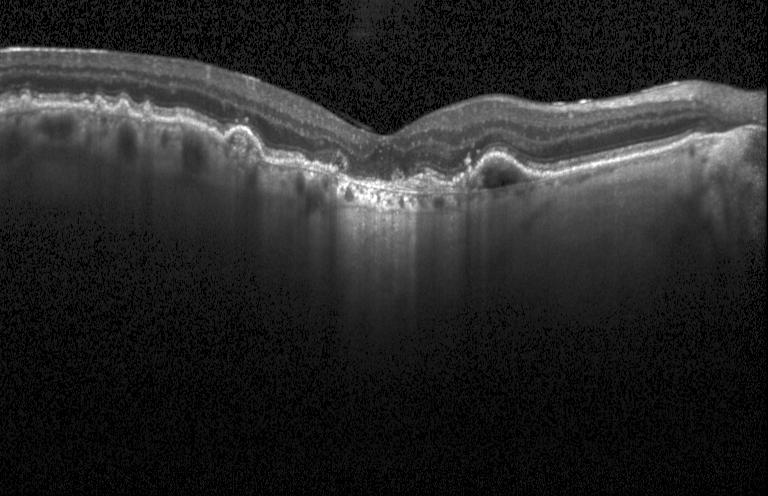 Spectral-domain optical coherence tomography. Heidelberg Spectralis. Macular scan. Optical coherence tomography scan. Diagnosis: a choroidal neovascular membrane.